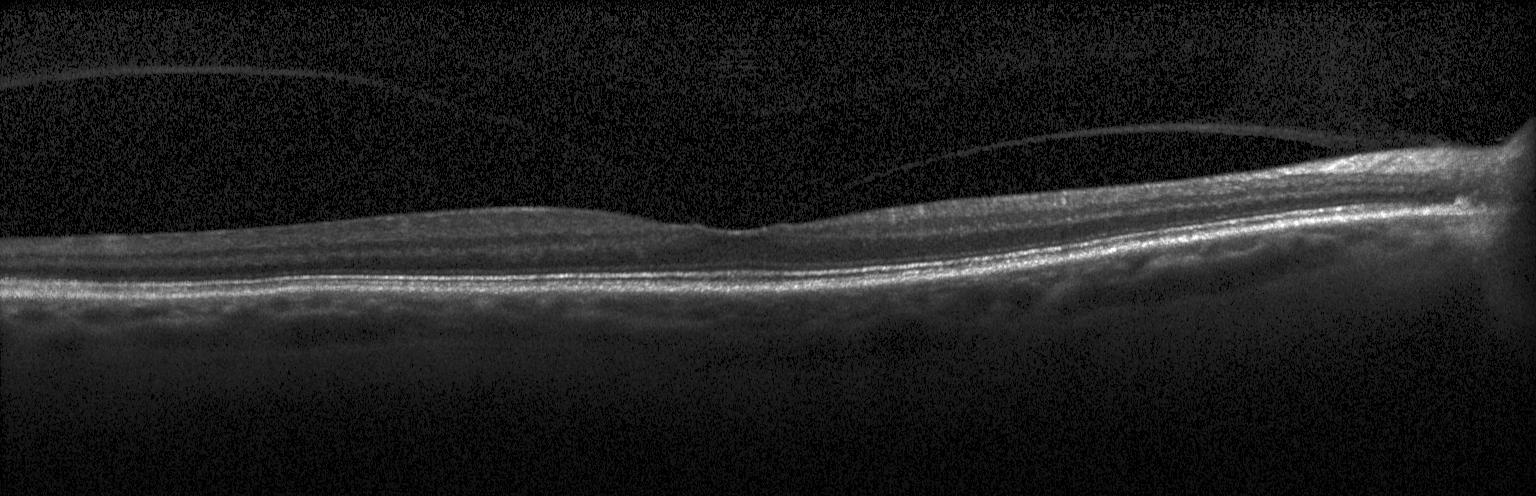 OCT finding: neither CNV, DME, nor drusen.